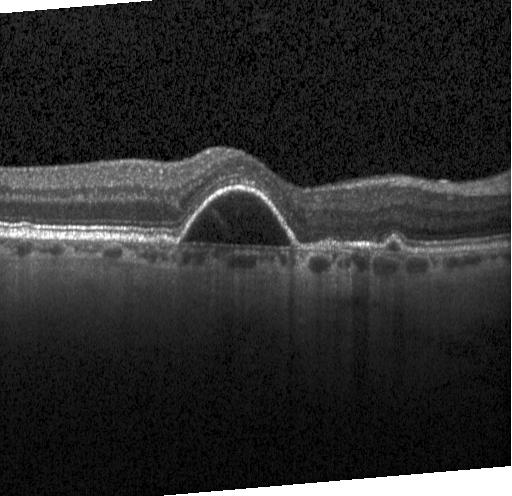
Through the macula; spectral-domain optical coherence tomography; retinal OCT B-scan — The scan shows CNV.